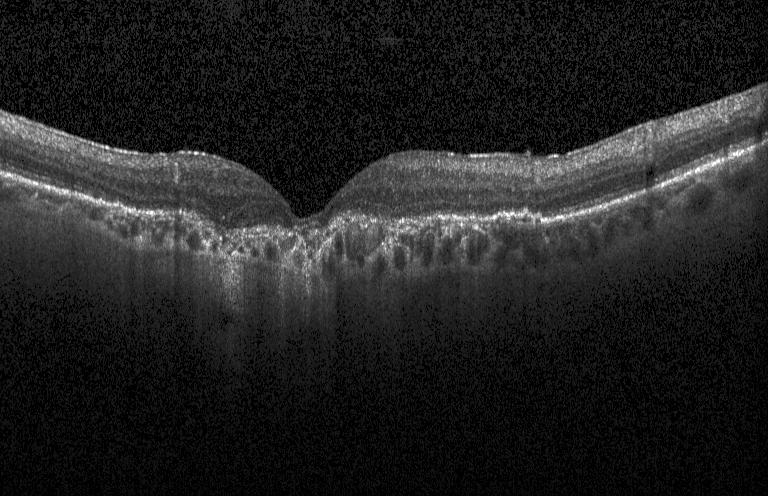
OCT scan showing a choroidal neovascular membrane.